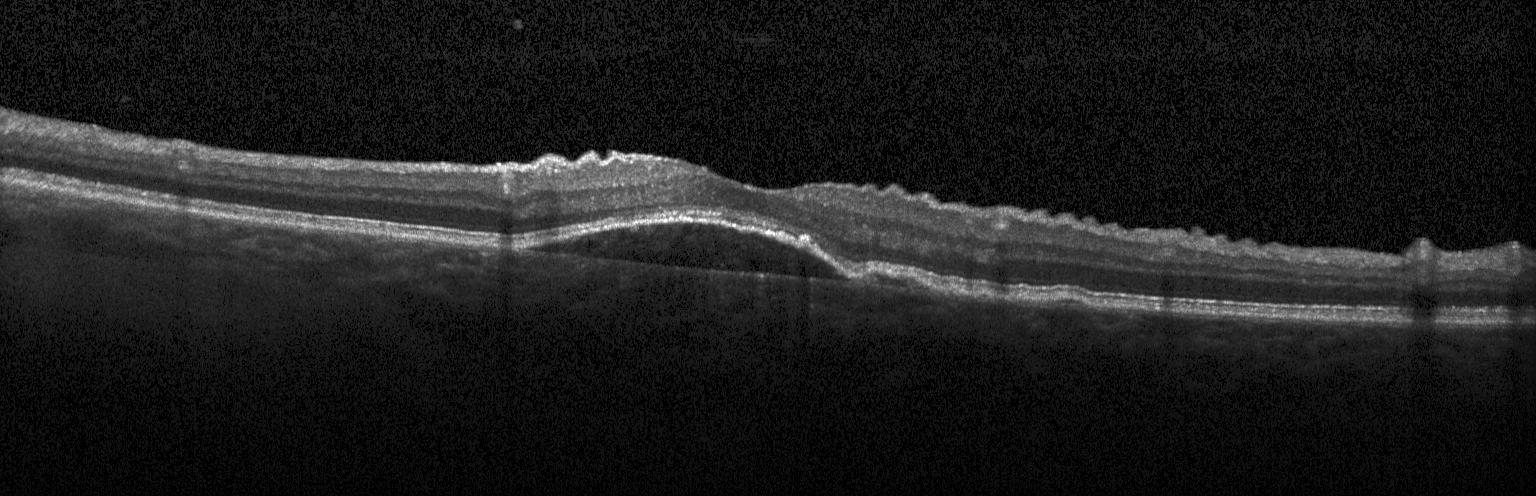 OCT line scan.
Finding: choroidal neovascularization (CNV).